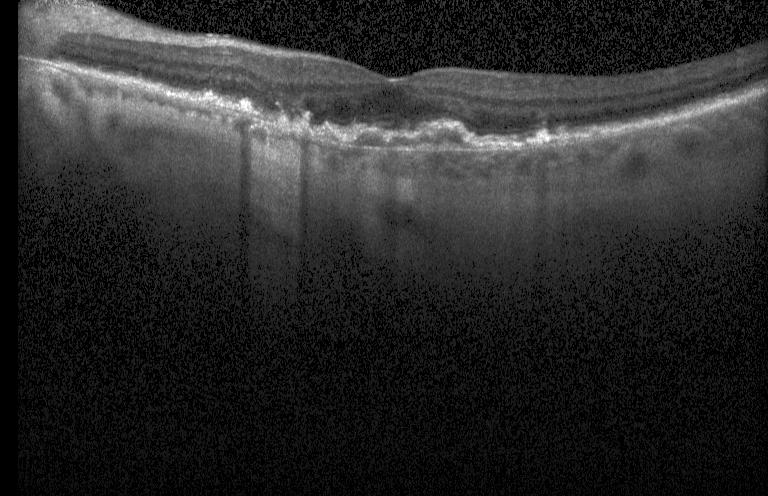 Assessment: a choroidal neovascular membrane.